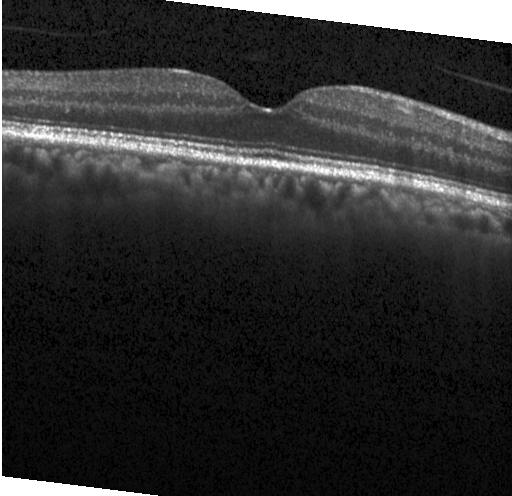 OCT B-scan showing no evidence of choroidal neovascularization, diabetic macular edema, or drusen.